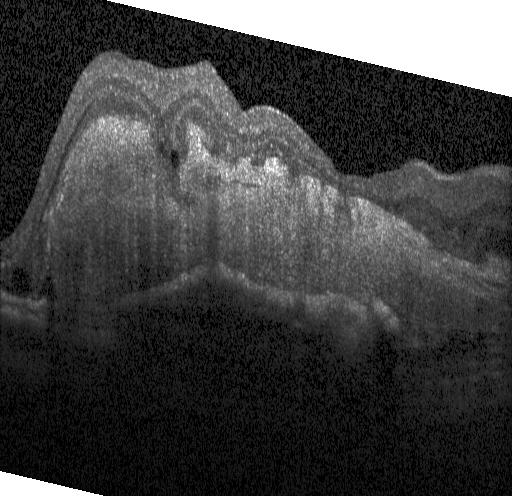 Spectral-domain OCT; optical coherence tomography scan.
A choroidal neovascular membrane.